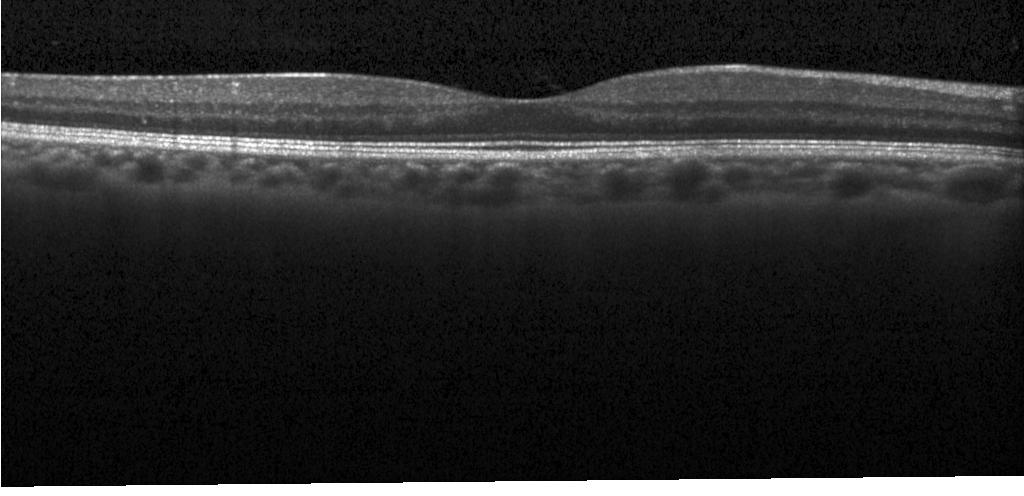 Optical coherence tomography scan; through the macula. Dx: no evidence of CNV, DME, or drusen.